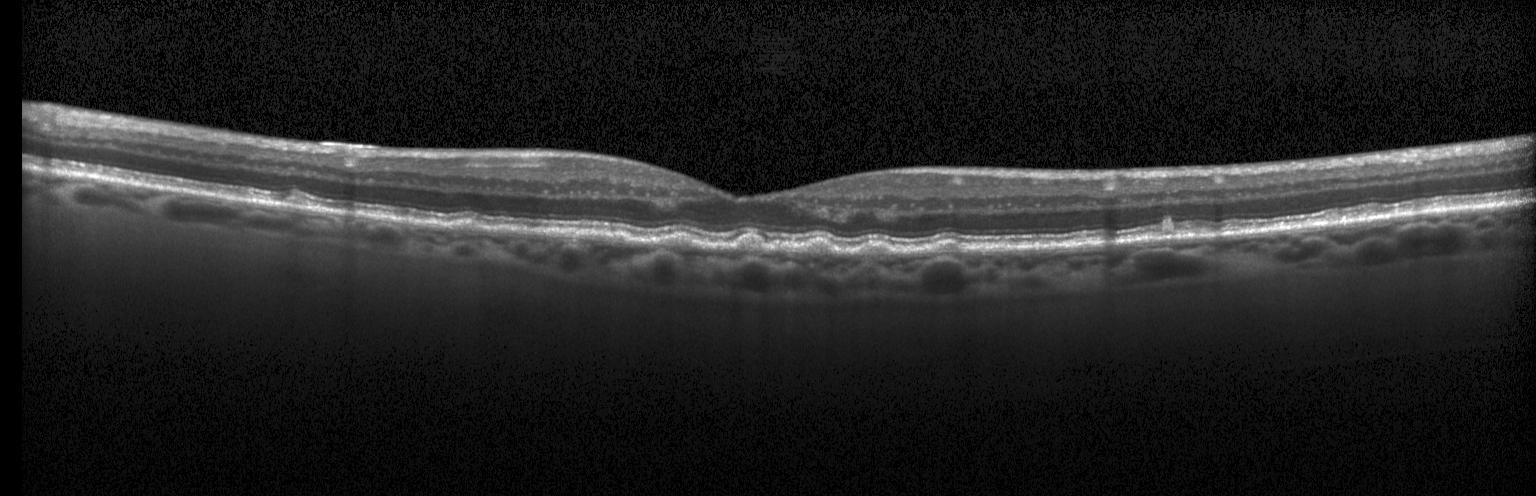

Optical coherence tomography B-scan.
Multiple drusen.